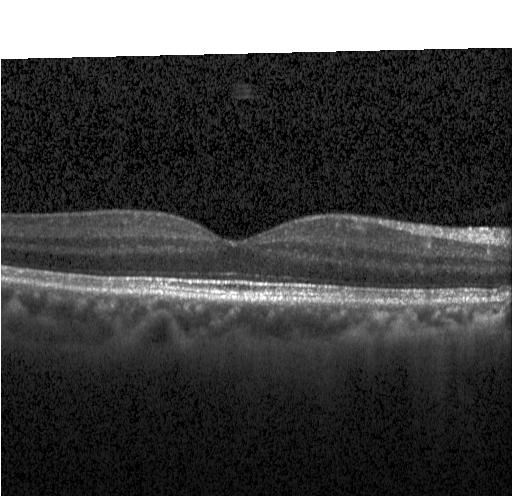 Instrument: Heidelberg Spectralis · macular scan · retinal OCT B-scan. This B-scan demonstrates no choroidal neovascularization, no diabetic macular edema, and no drusen.